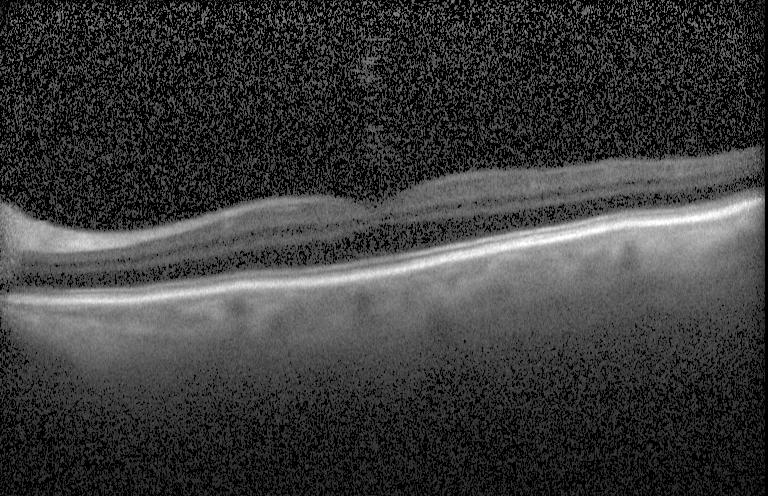
Dx: no evidence of choroidal neovascularization, diabetic macular edema, or drusen.